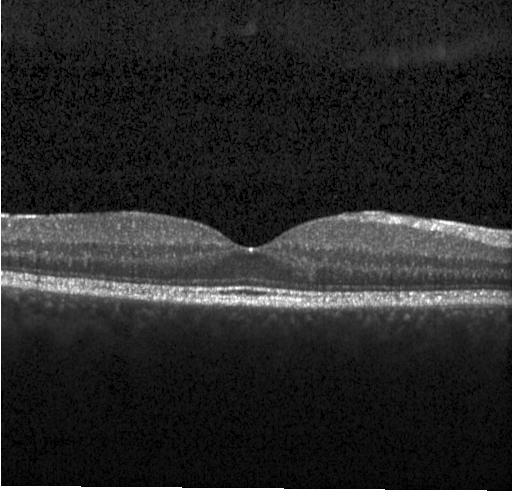 OCT scan showing no choroidal neovascularization, diabetic macular edema, or drusen.